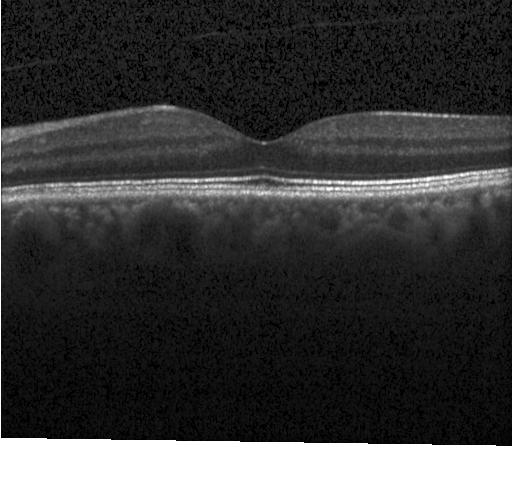

OCT scan showing neither CNV, DME, nor drusen.